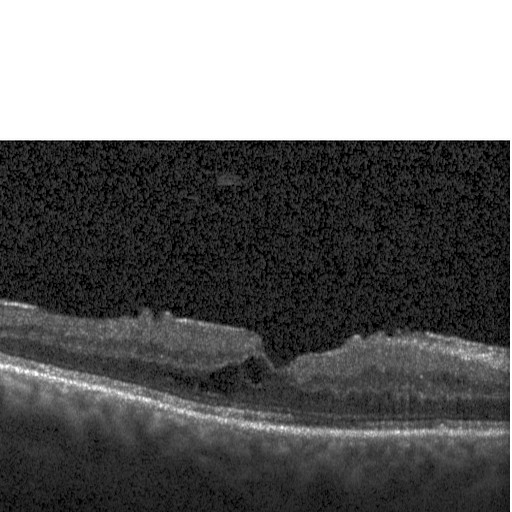

The scan shows DME.